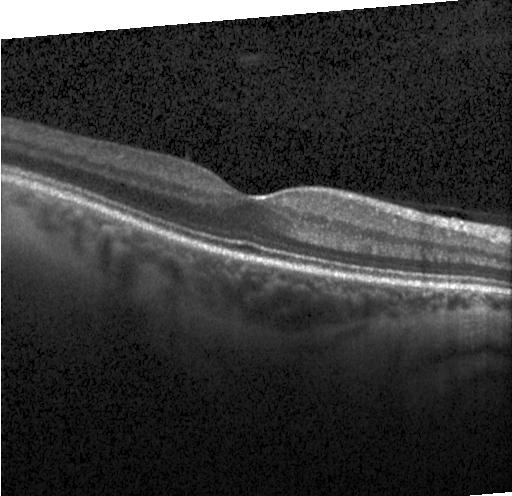
Retinal OCT B-scan · Heidelberg Spectralis OCT system
Impression: no evidence of choroidal neovascularization, diabetic macular edema, or drusen.